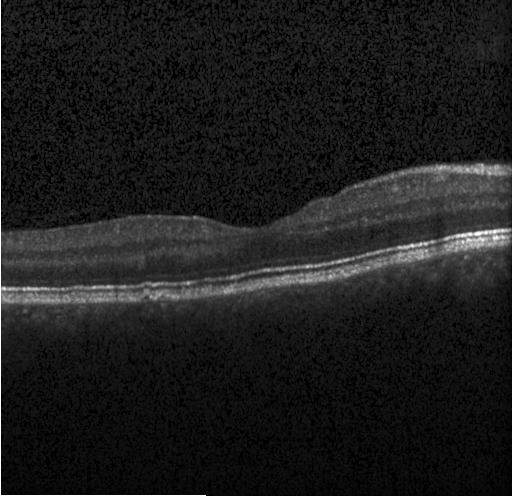 Retinal OCT B-scan
Diagnosis: no CNV, DME, or drusen.